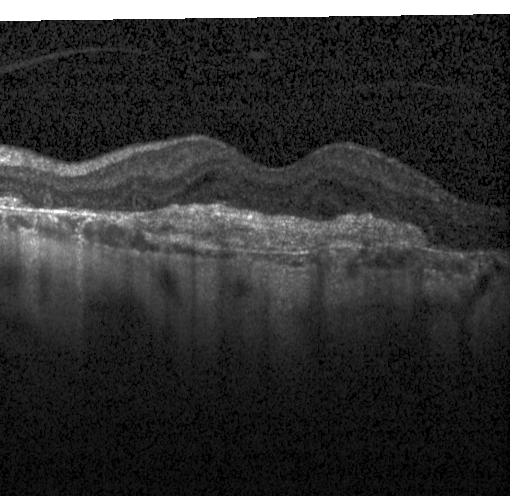
Impression: choroidal neovascularization.